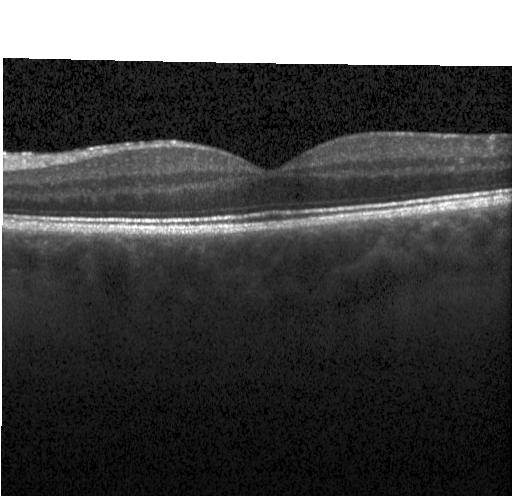

Spectral-domain OCT · OCT B-scan · fovea-centered · Heidelberg Spectralis OCT system.
Impression: no choroidal neovascularization, diabetic macular edema, or drusen.